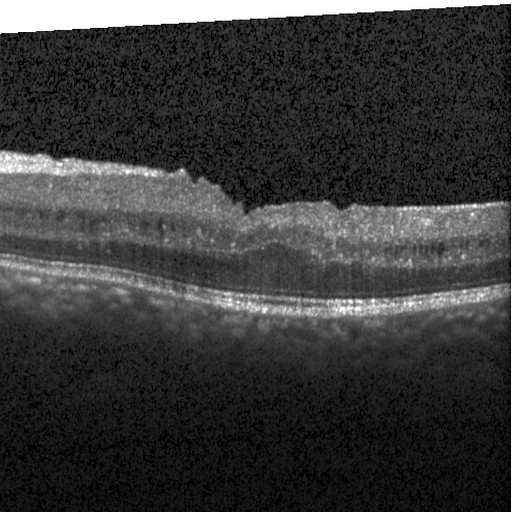 OCT B-scan showing diabetic macular edema.